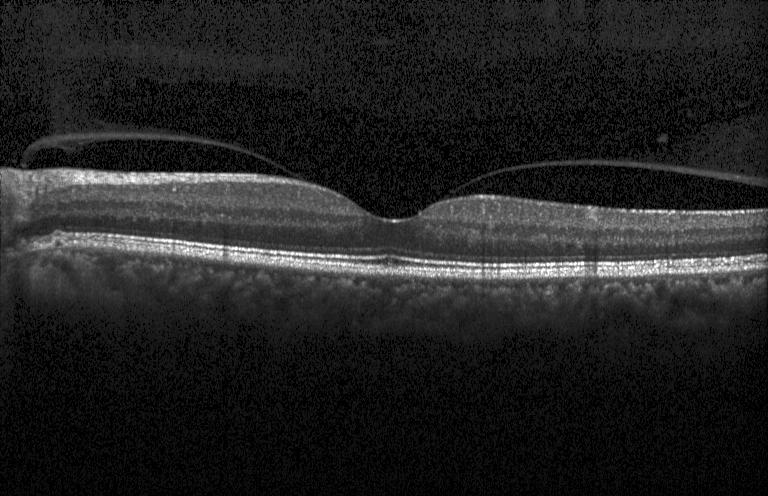 OCT finding: no evidence of choroidal neovascularization, diabetic macular edema, or drusen.